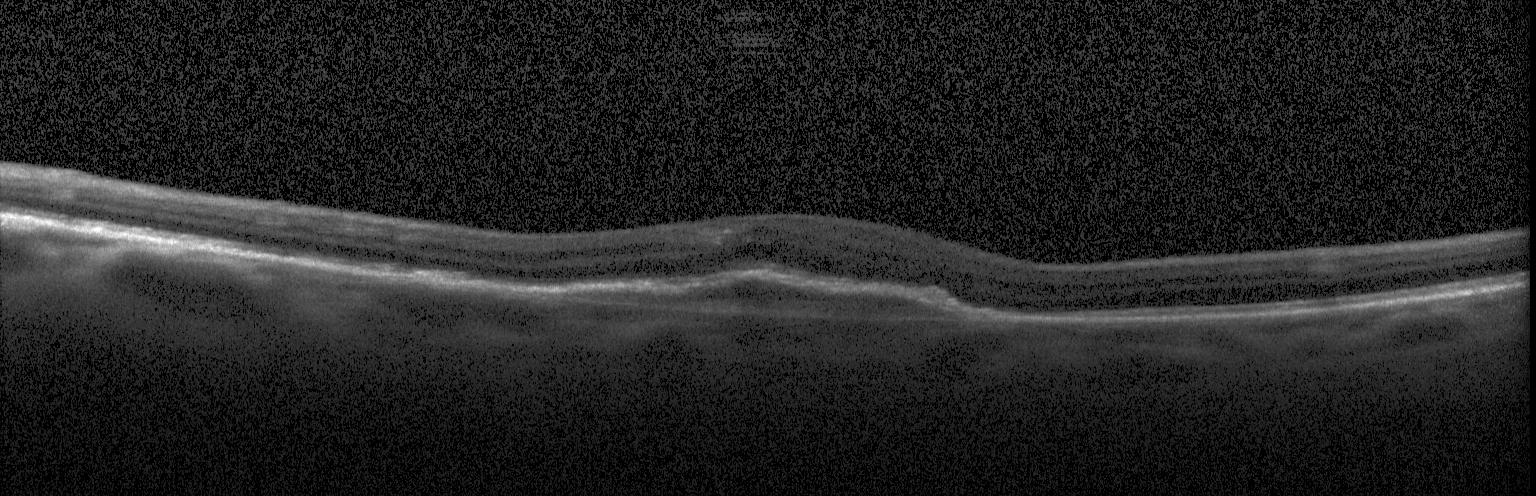 Optical coherence tomography scan. Macular OCT: a choroidal neovascular membrane.